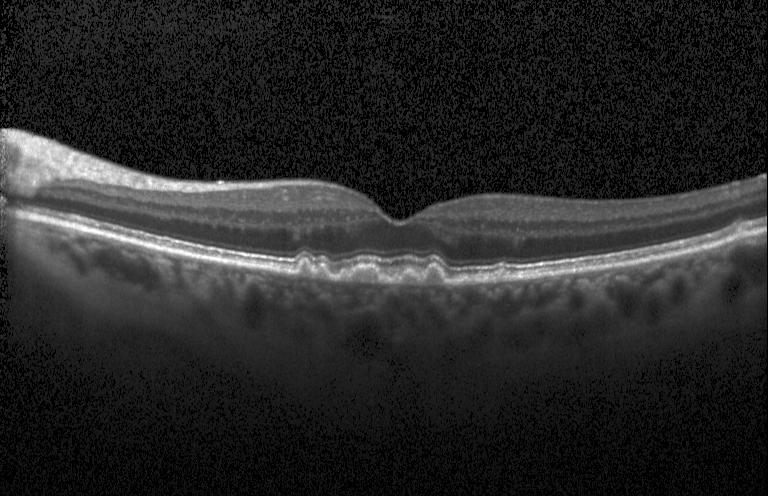
OCT line scan; macular scan; acquired on a Heidelberg Spectralis; spectral-domain OCT. OCT finding: sub-RPE drusenoid deposits.